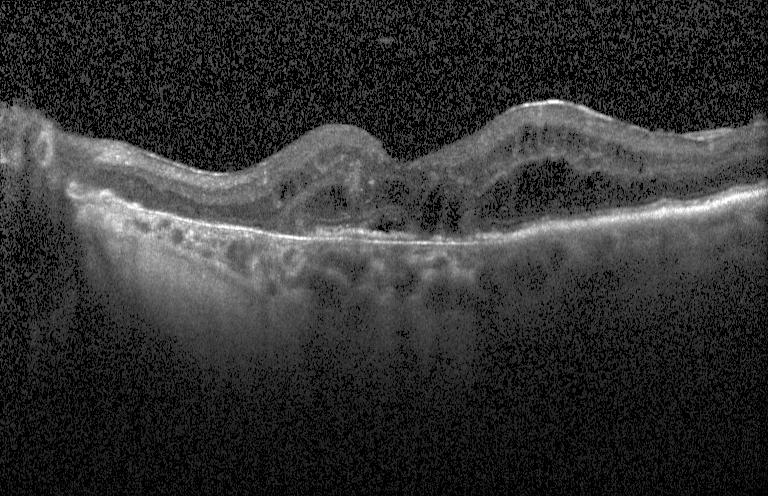 Spectral-domain OCT B-scan: a choroidal neovascular membrane.